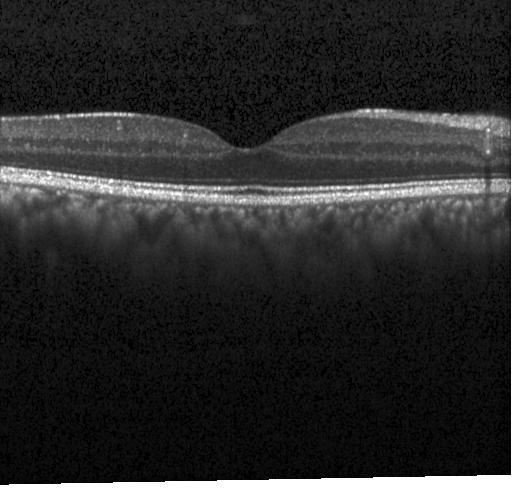 Macular scan, Heidelberg Spectralis, optical coherence tomography scan.
Diagnosis: no choroidal neovascularization, diabetic macular edema, or drusen.